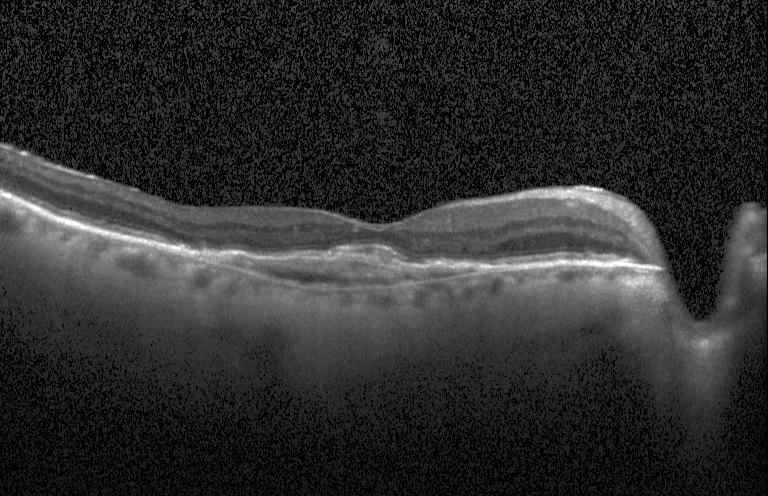
Spectral-domain optical coherence tomography, retinal OCT cross-section, Heidelberg Spectralis. OCT finding: a choroidal neovascular membrane.